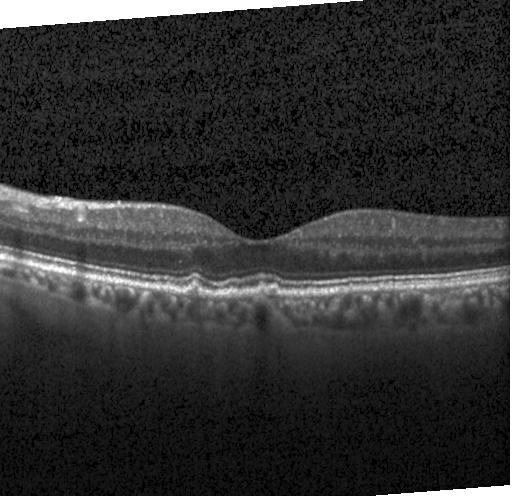

Spectral-domain OCT B-scan: drusen.